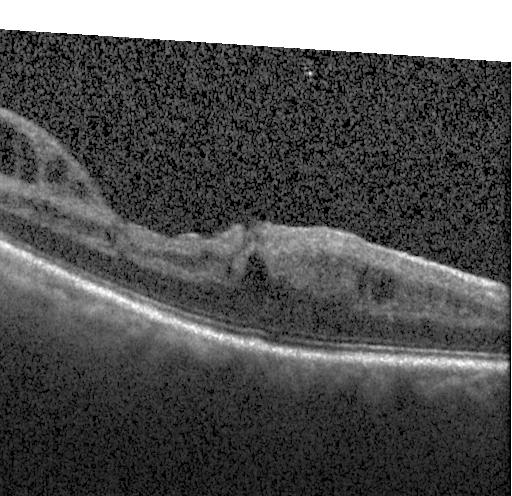
OCT scan showing DME.